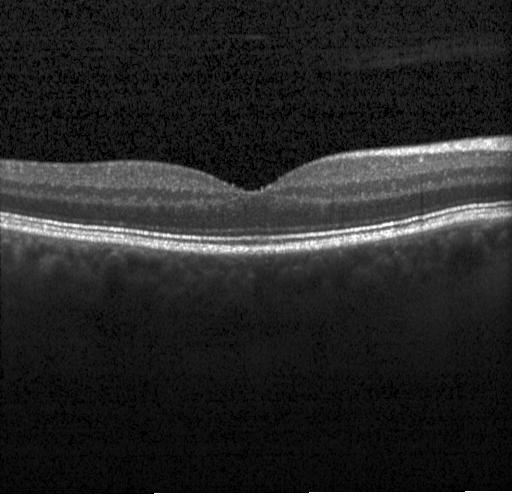
Centered on the fovea. SD-OCT. Optical coherence tomography B-scan
Finding: no choroidal neovascularization, diabetic macular edema, or drusen.